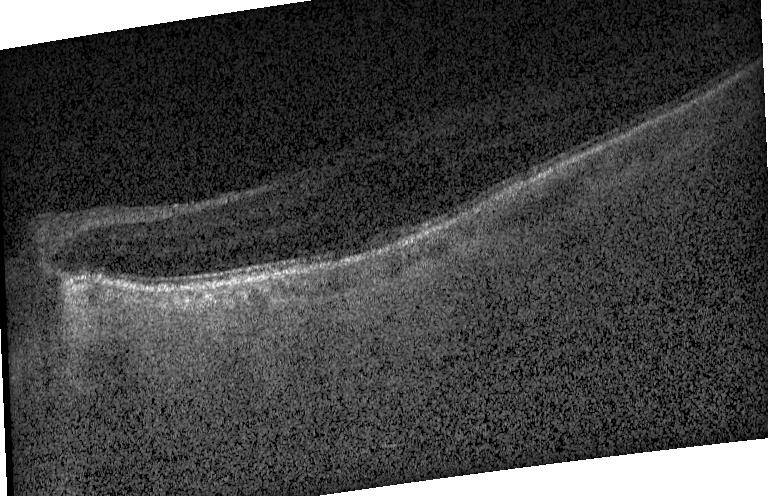

Retinal OCT cross-section showing diabetic macular edema.